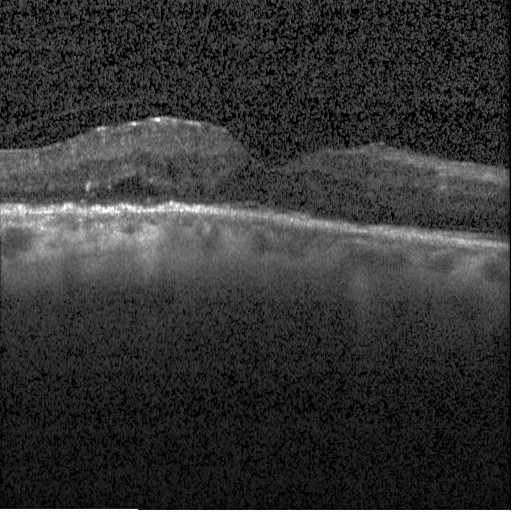 Optical coherence tomography scan.
Diagnosis: diabetic macular edema.